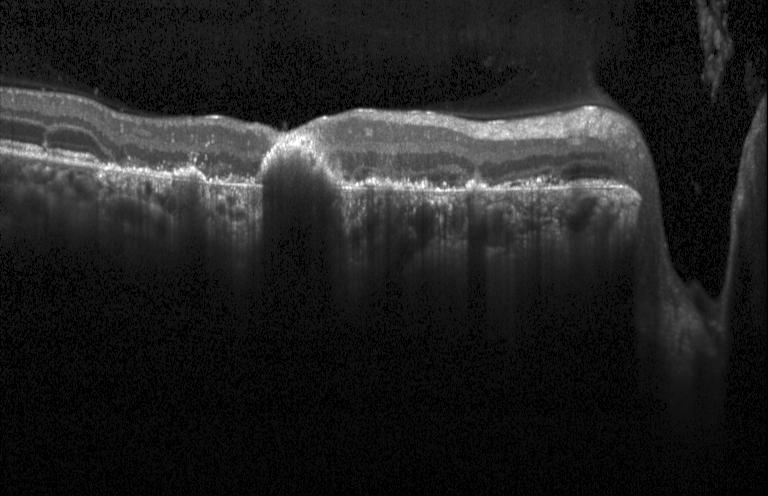 Optical coherence tomography B-scan; macular scan. Assessment: choroidal neovascularization (CNV).